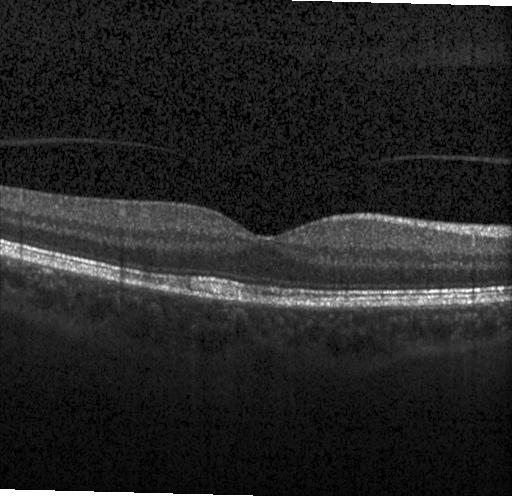 Impression: no choroidal neovascularization, no diabetic macular edema, and no drusen.